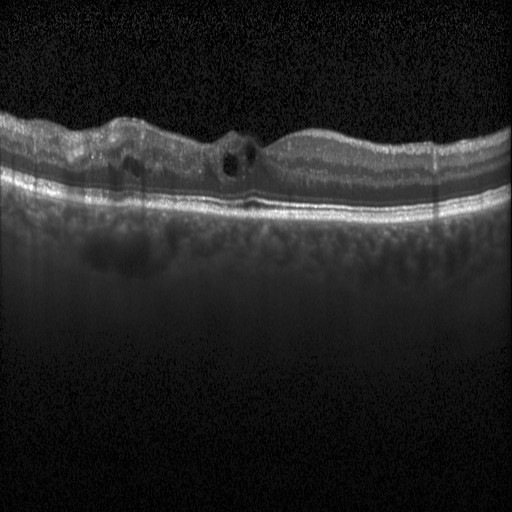

Instrument: Heidelberg Spectralis, spectral-domain OCT, optical coherence tomography scan — Impression: diabetic macular edema.